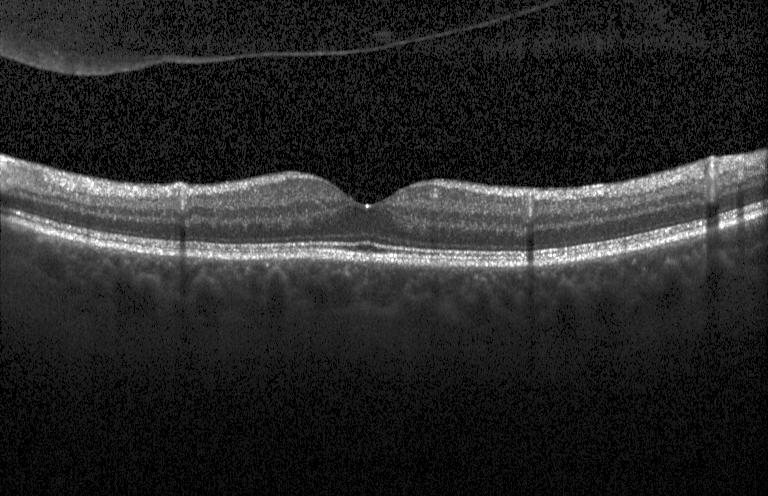
The scan shows no evidence of choroidal neovascularization, diabetic macular edema, or drusen.